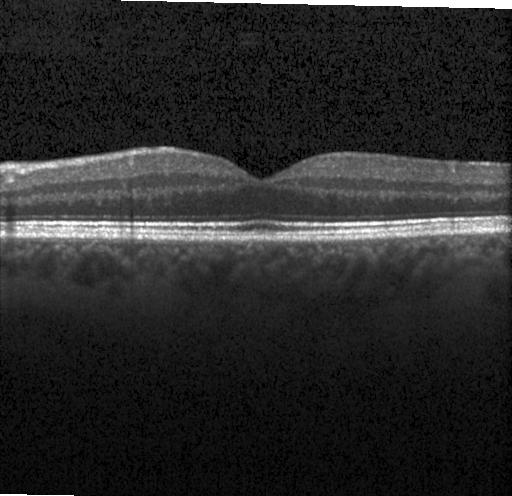

Acquired on a Heidelberg Spectralis · fovea-centered · retinal OCT B-scan · spectral-domain optical coherence tomography
Neither CNV, DME, nor drusen.